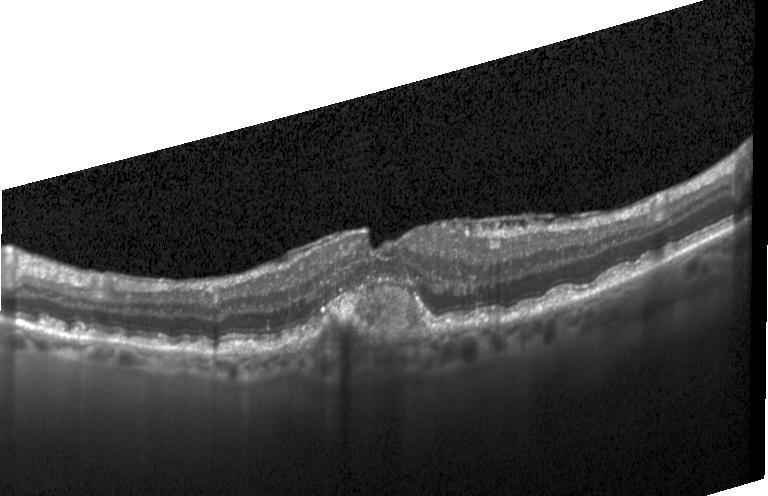
Heidelberg Spectralis OCT system; OCT line scan. Assessment: choroidal neovascularization (CNV).